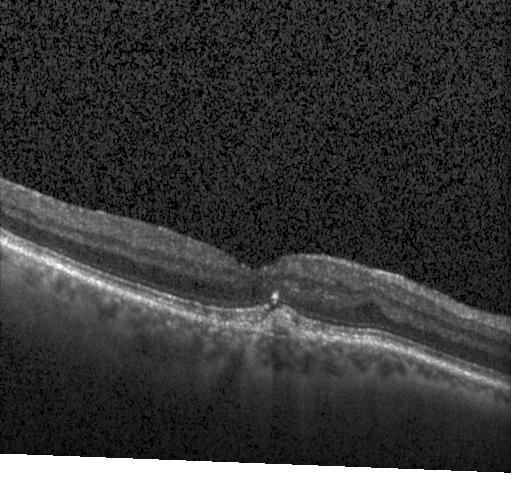

Impression: a choroidal neovascular membrane.